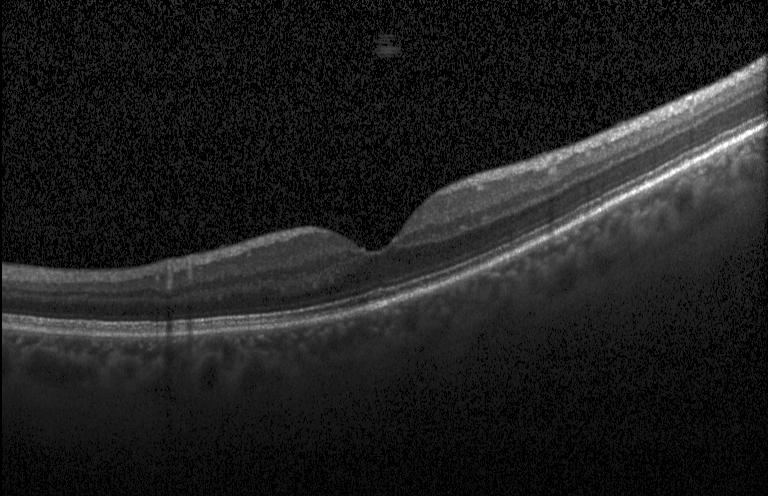
Optical coherence tomography B-scan. Acquired on a Heidelberg Spectralis. Spectral-domain optical coherence tomography. The scan shows no choroidal neovascularization, diabetic macular edema, or drusen.